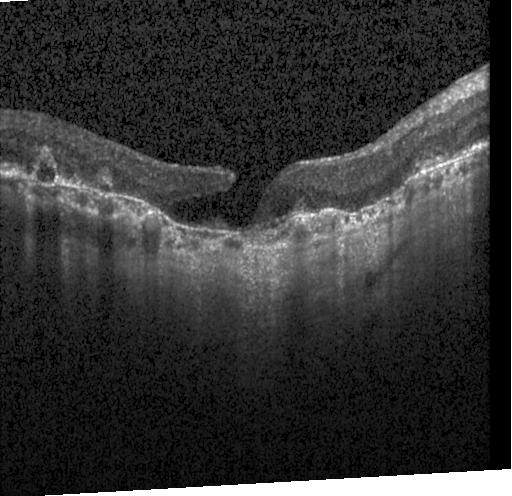
OCT scan showing a choroidal neovascular membrane.